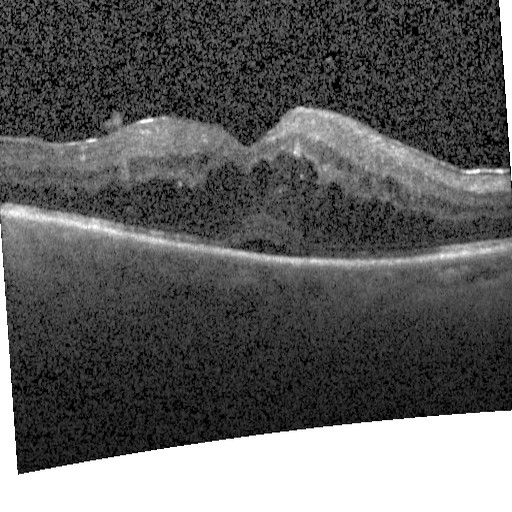

This B-scan demonstrates diabetic macular edema.